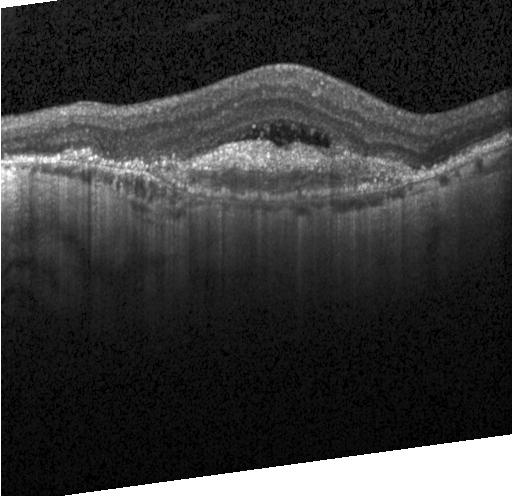 Instrument: Heidelberg Spectralis; SD-OCT; OCT B-scan; through the macula — Impression: a choroidal neovascular membrane.